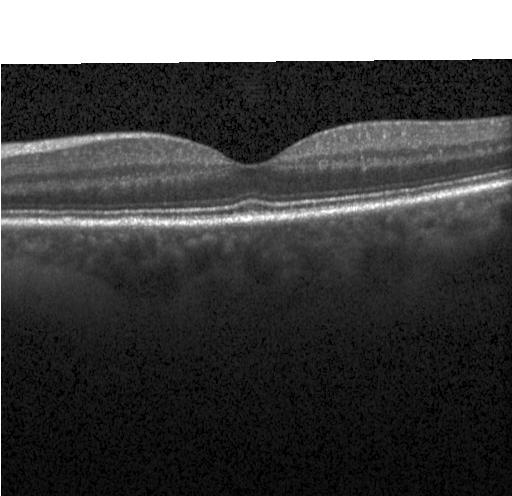

Macular OCT demonstrating no choroidal neovascularization, diabetic macular edema, or drusen.